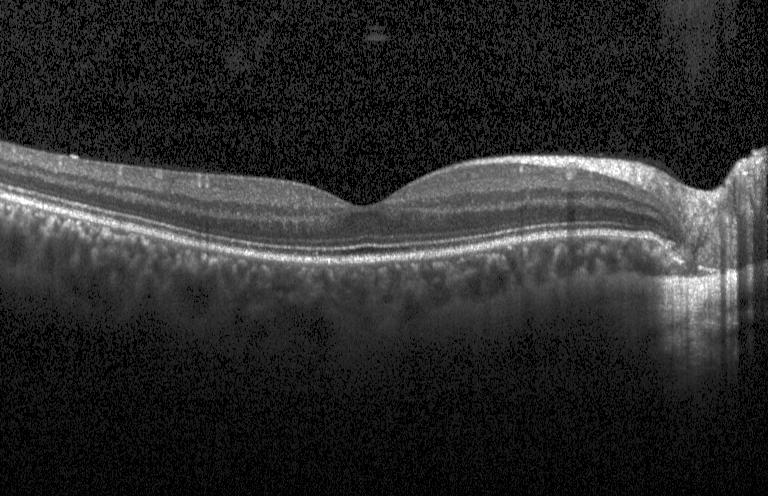
OCT B-scan showing no evidence of choroidal neovascularization, diabetic macular edema, or drusen.